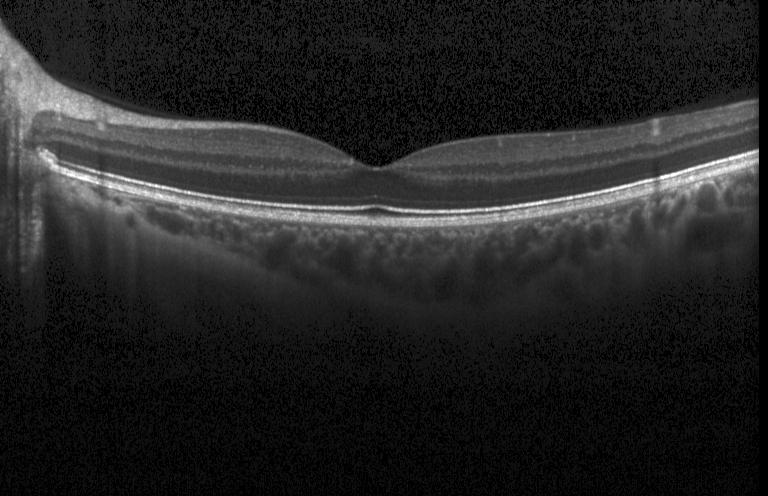
SD-OCT; optical coherence tomography B-scan; macular scan
Diagnosis: no choroidal neovascularization, diabetic macular edema, or drusen.